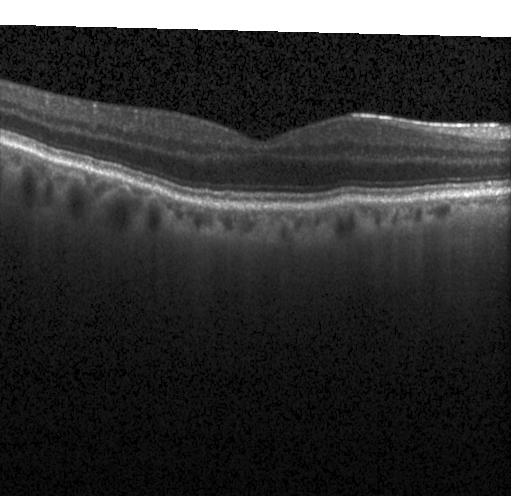
Instrument: Heidelberg Spectralis · OCT line scan · spectral-domain optical coherence tomography
Finding: no choroidal neovascularization, no diabetic macular edema, and no drusen.